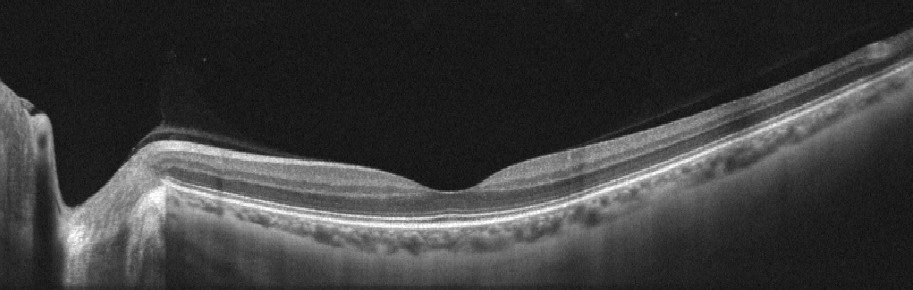 Optovue Avanti RTVue XR; OCT B-scan. No AMD, DME, ERM, RAO, RVO, or VID.